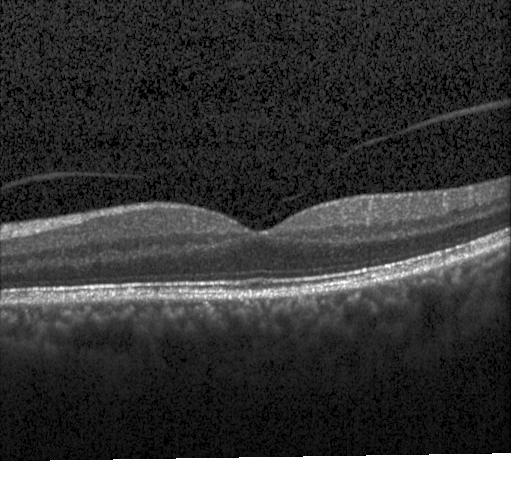

Fovea-centered; optical coherence tomography B-scan.
Finding: neither choroidal neovascularization, diabetic macular edema, nor drusen.